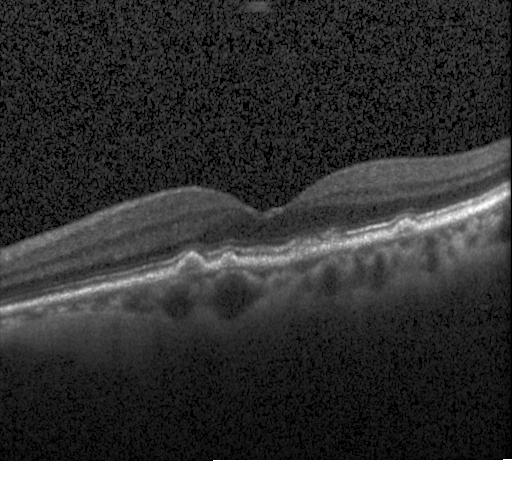 Retinal OCT cross-section showing sub-RPE drusenoid deposits.